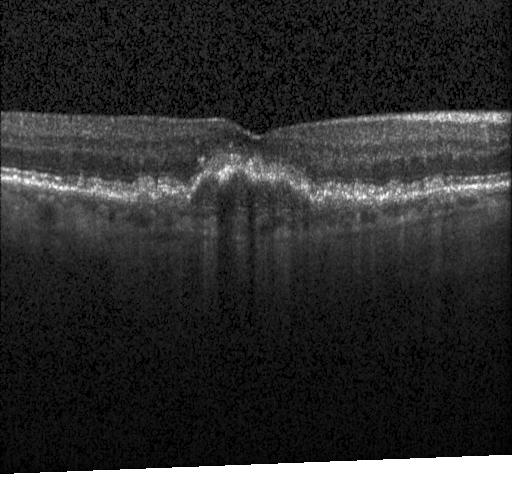
Finding: a choroidal neovascular membrane.